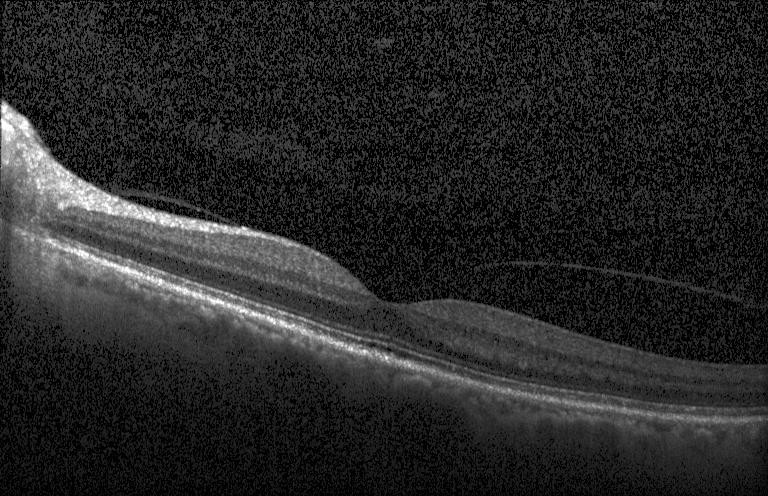

Horizontal scan through the fovea, optical coherence tomography scan, Heidelberg Spectralis — Finding: no choroidal neovascularization, diabetic macular edema, or drusen.